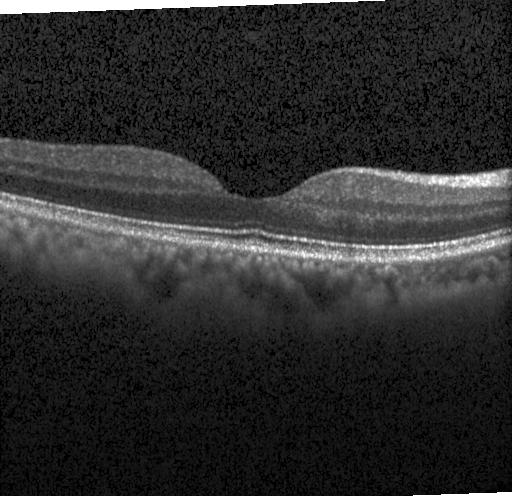 Finding: no evidence of choroidal neovascularization, diabetic macular edema, or drusen.